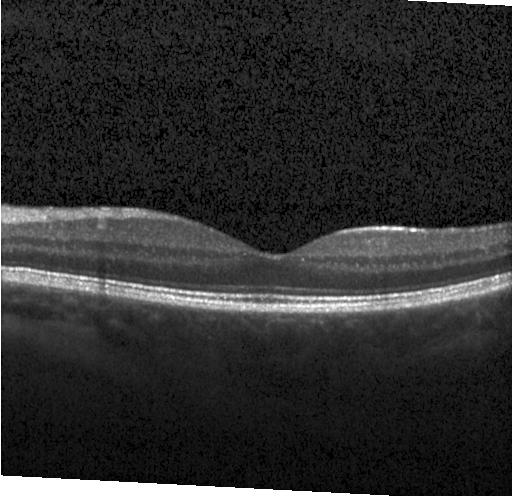
Optical coherence tomography scan. Heidelberg Spectralis. Horizontal scan through the fovea — OCT finding: neither CNV, DME, nor drusen.